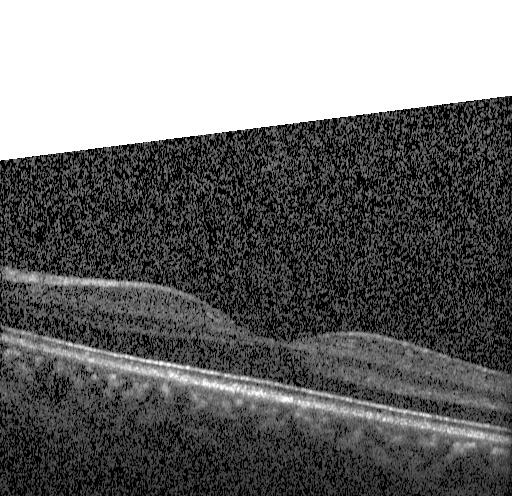

OCT B-scan showing no evidence of CNV, DME, or drusen.